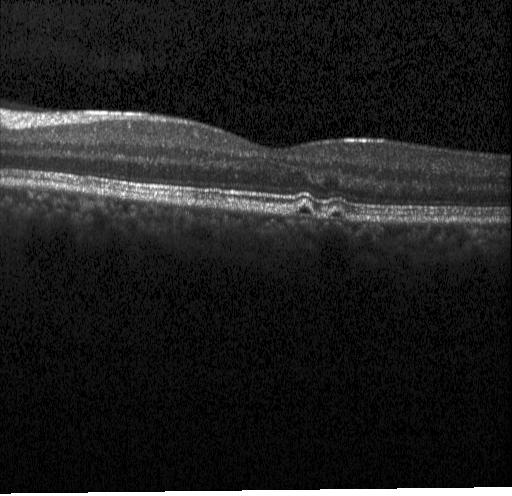

OCT scan showing drusen.